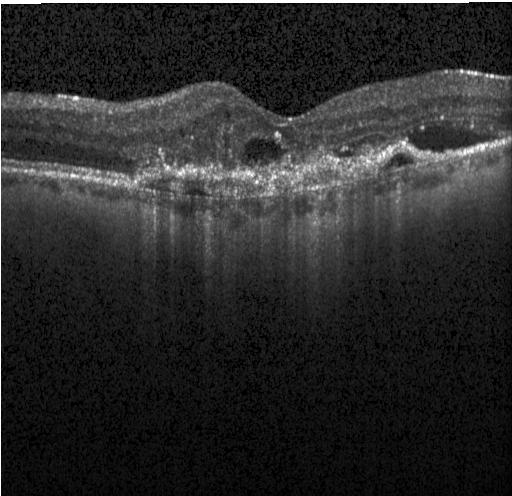
Finding: a choroidal neovascular membrane.